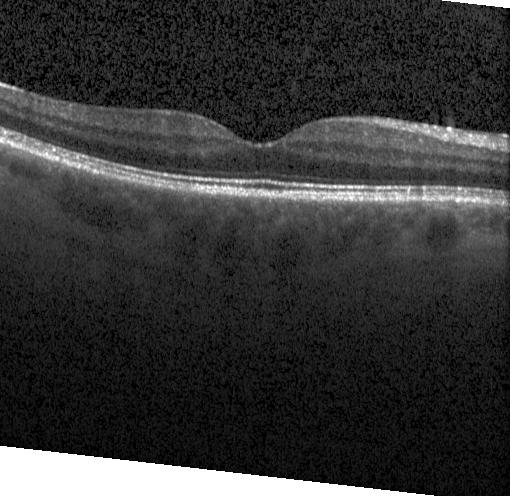 Through the macula, spectral-domain OCT, retinal OCT B-scan
This B-scan demonstrates no evidence of CNV, DME, or drusen.